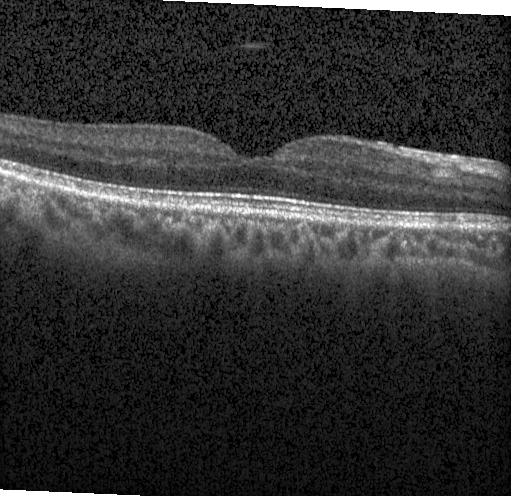

Optical coherence tomography scan, acquired on a Heidelberg Spectralis, spectral-domain optical coherence tomography
Assessment: no CNV, DME, or drusen.